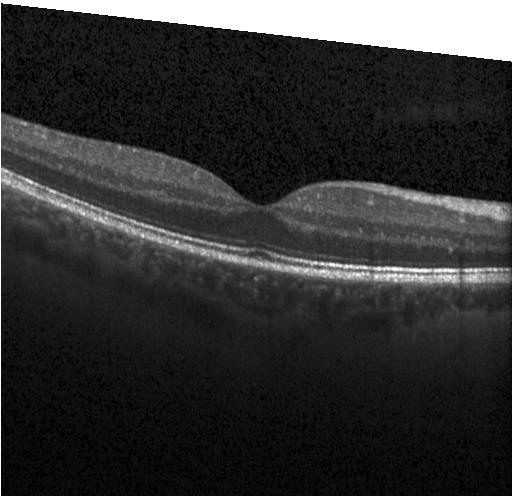
Impression: no evidence of choroidal neovascularization, diabetic macular edema, or drusen.